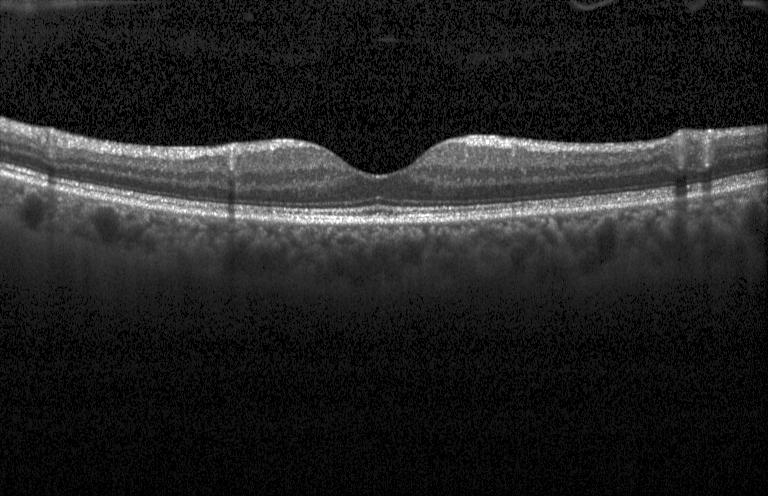 Optical coherence tomography scan · Heidelberg Spectralis OCT system
The scan shows neither CNV, DME, nor drusen.